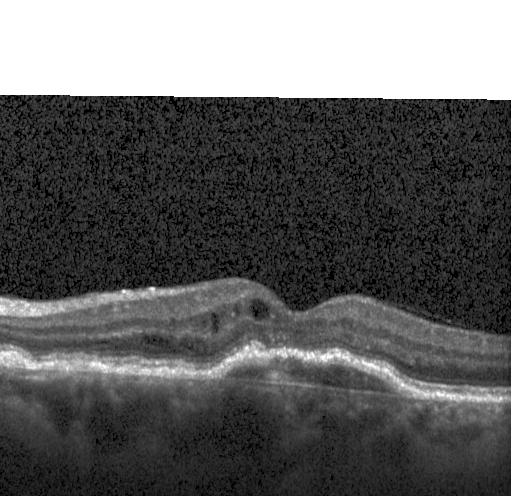

Spectral-domain OCT B-scan: a choroidal neovascular membrane.